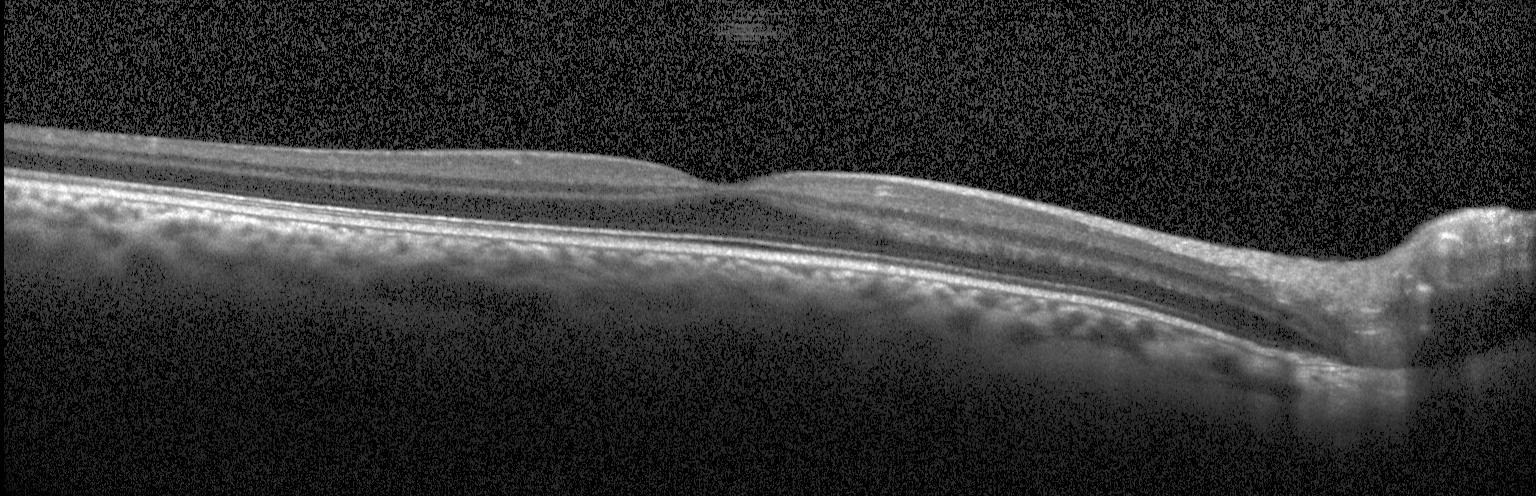 Instrument: Heidelberg Spectralis, OCT B-scan.
Diagnosis: neither choroidal neovascularization, diabetic macular edema, nor drusen.